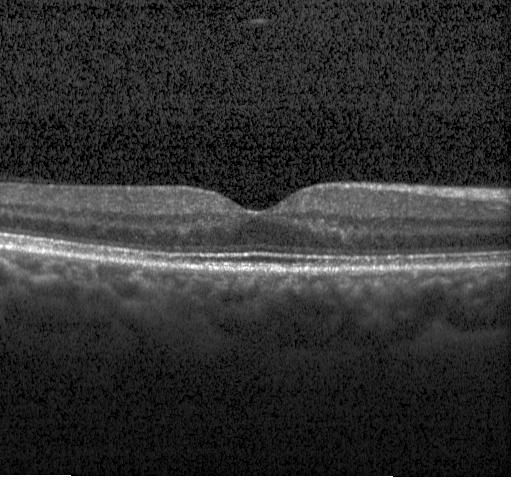
Diagnosis: neither CNV, DME, nor drusen.